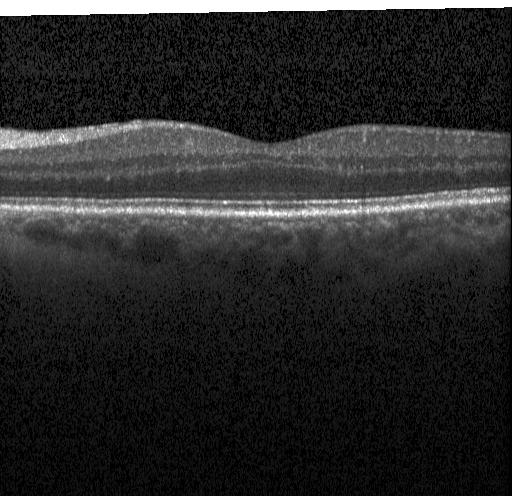
Macular OCT demonstrating no evidence of choroidal neovascularization, diabetic macular edema, or drusen.